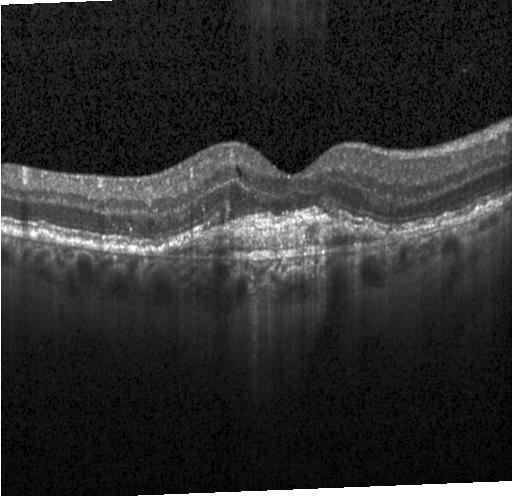
Dx: choroidal neovascularization (CNV).